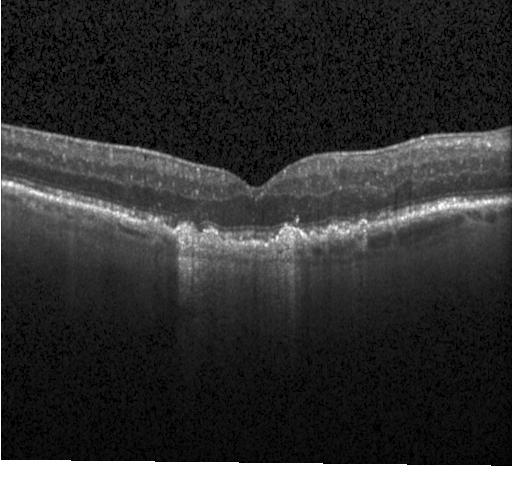 OCT B-scan
The scan shows a choroidal neovascular membrane.